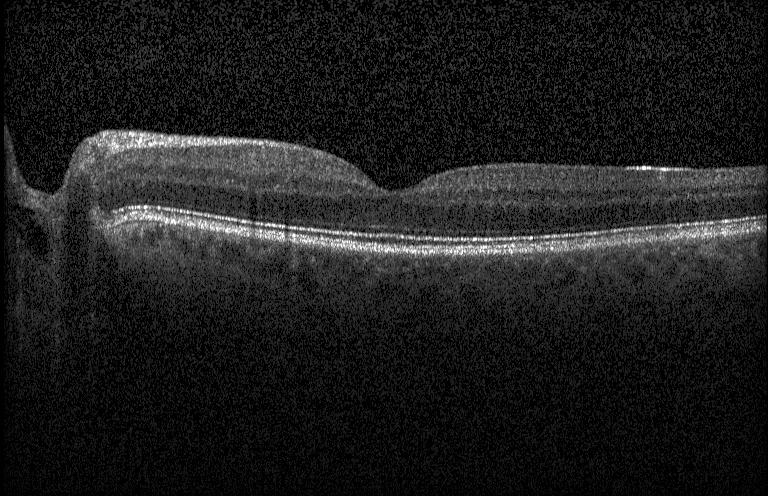

Finding: no choroidal neovascularization, diabetic macular edema, or drusen.